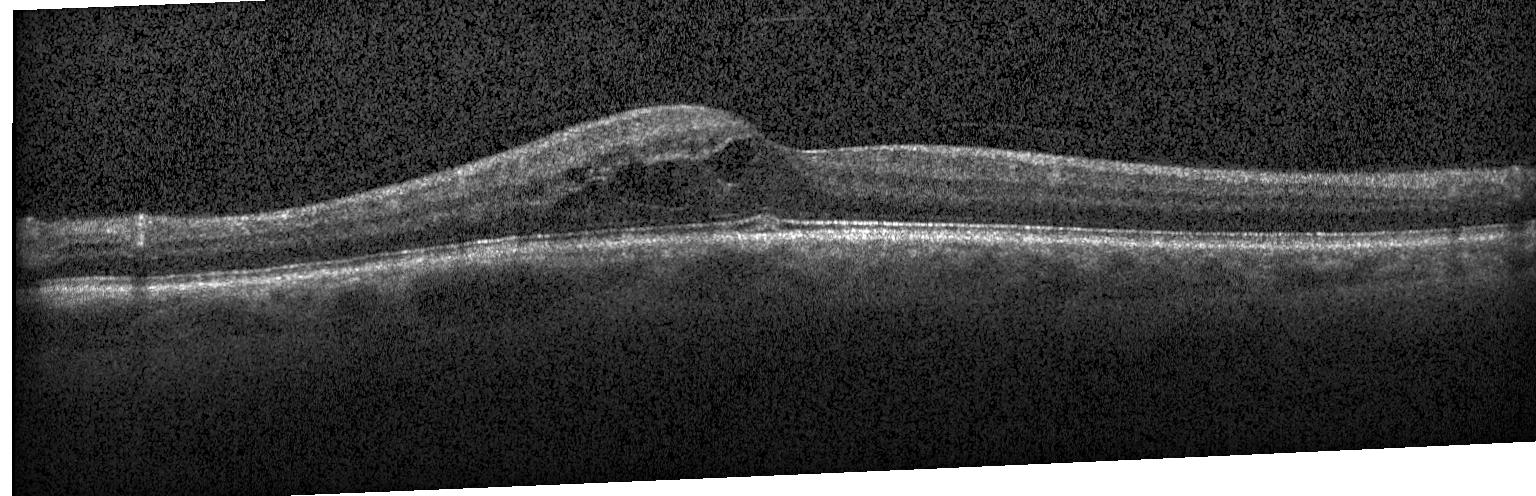
Impression: DME.